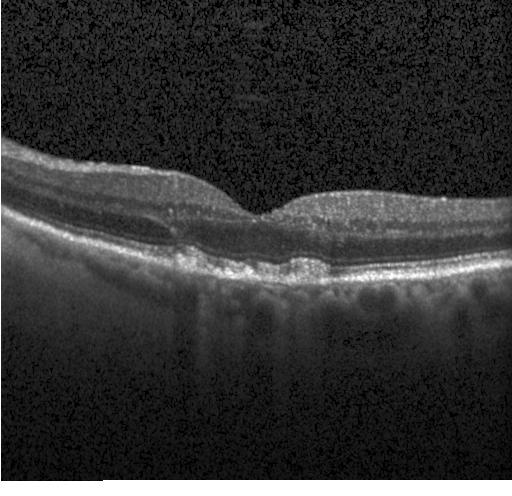

The scan shows sub-RPE drusenoid deposits.